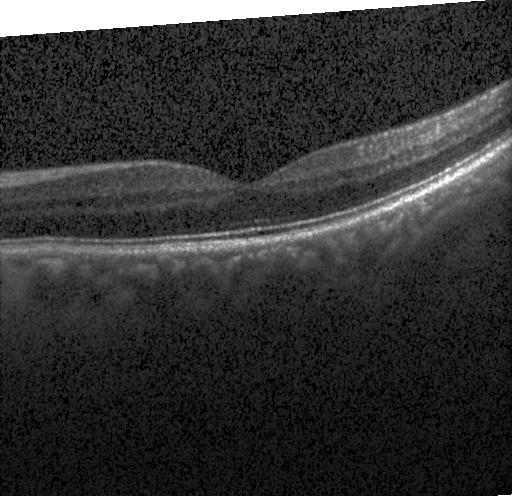 OCT B-scan showing neither CNV, DME, nor drusen.